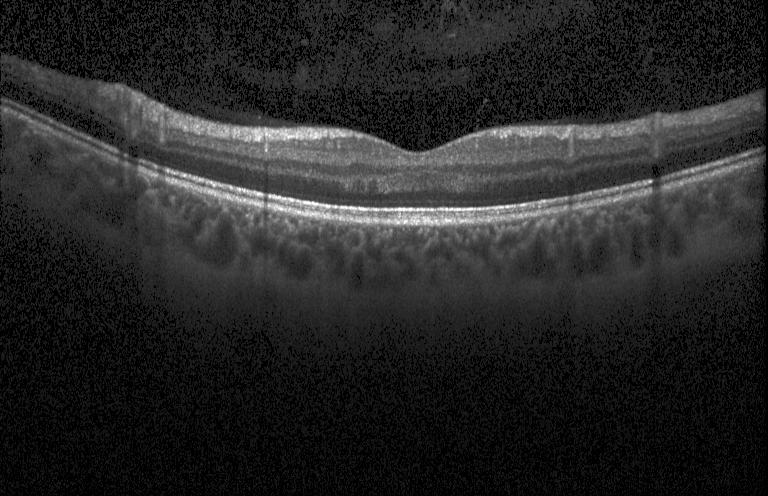
Horizontal scan through the fovea; OCT B-scan
Diagnosis: no CNV, DME, or drusen.